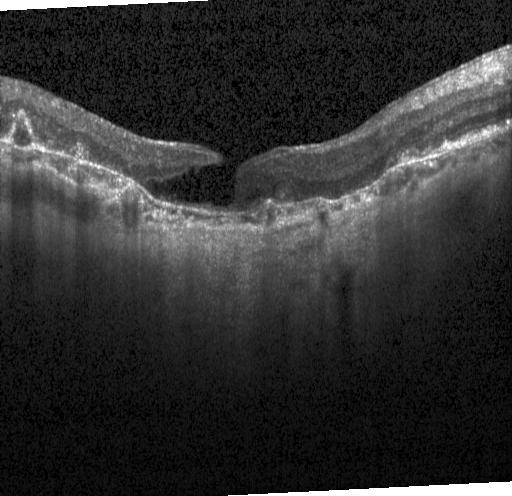

Diagnosis: choroidal neovascularization (CNV).